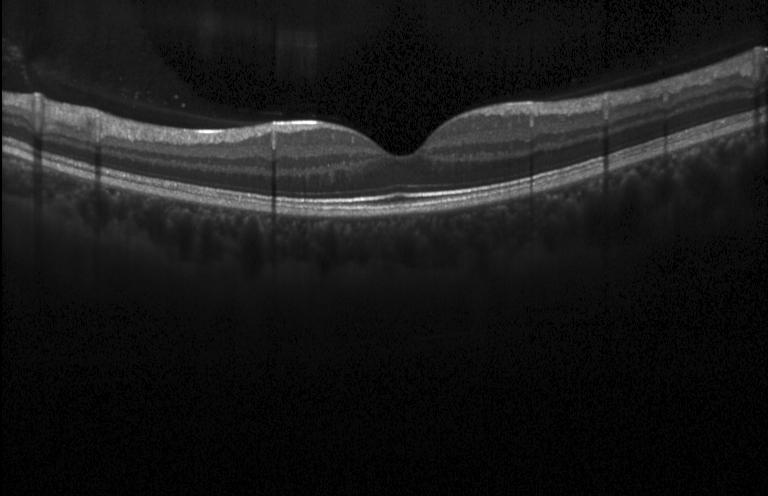 Finding: neither choroidal neovascularization, diabetic macular edema, nor drusen.